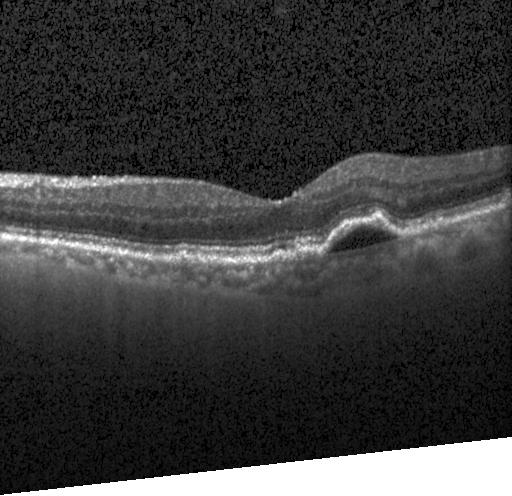 This B-scan demonstrates choroidal neovascularization (CNV).